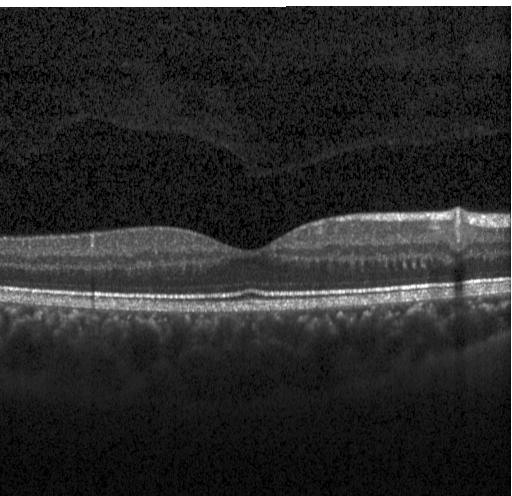
Centered on the fovea; spectral-domain OCT; Heidelberg Spectralis OCT system; retinal OCT cross-section. OCT finding: no choroidal neovascularization, diabetic macular edema, or drusen.